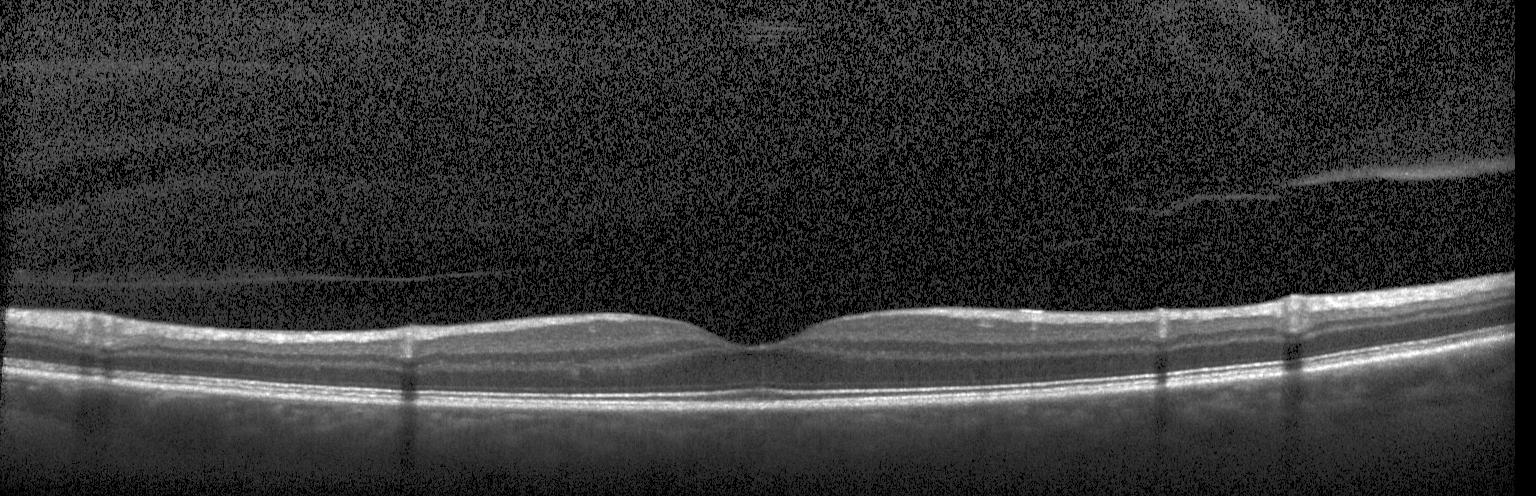

Heidelberg Spectralis OCT system. OCT line scan. Fovea-centered — OCT finding: no evidence of choroidal neovascularization, diabetic macular edema, or drusen.